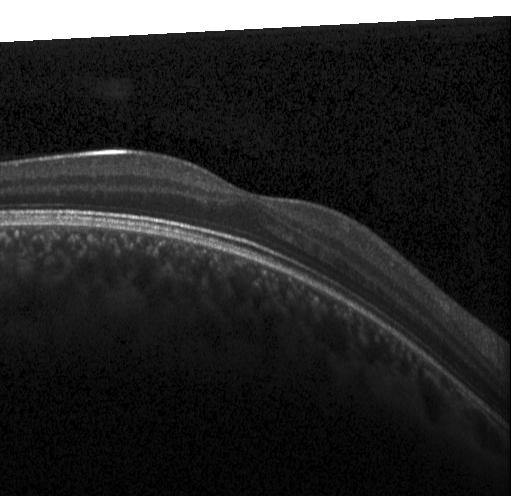

Macular OCT: neither choroidal neovascularization, diabetic macular edema, nor drusen.